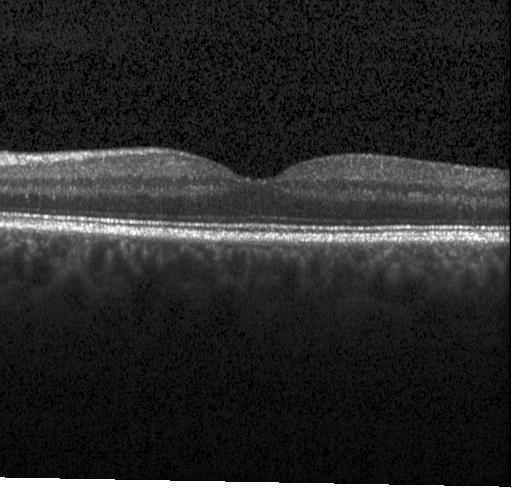

Impression: neither choroidal neovascularization, diabetic macular edema, nor drusen.